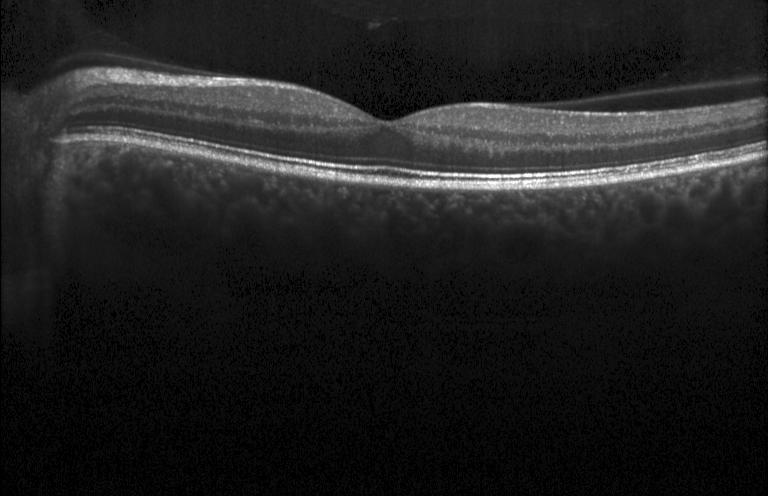

Heidelberg Spectralis, optical coherence tomography scan.
Assessment: no evidence of choroidal neovascularization, diabetic macular edema, or drusen.